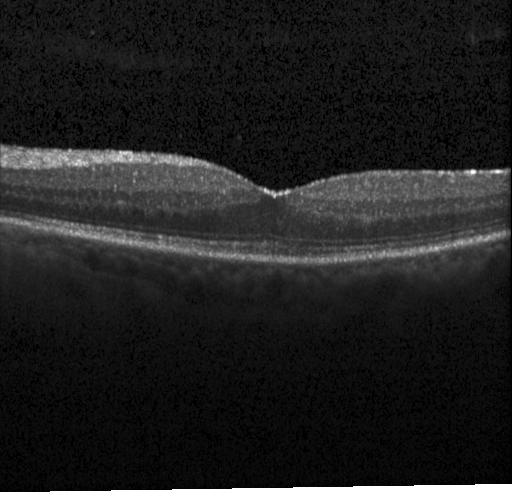
Retinal OCT B-scan, spectral-domain optical coherence tomography, fovea-centered. Impression: no choroidal neovascularization, diabetic macular edema, or drusen.